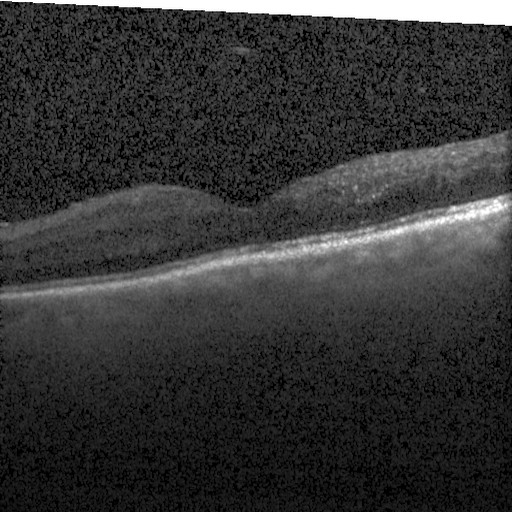

Retinal OCT cross-section.
This B-scan demonstrates DME.